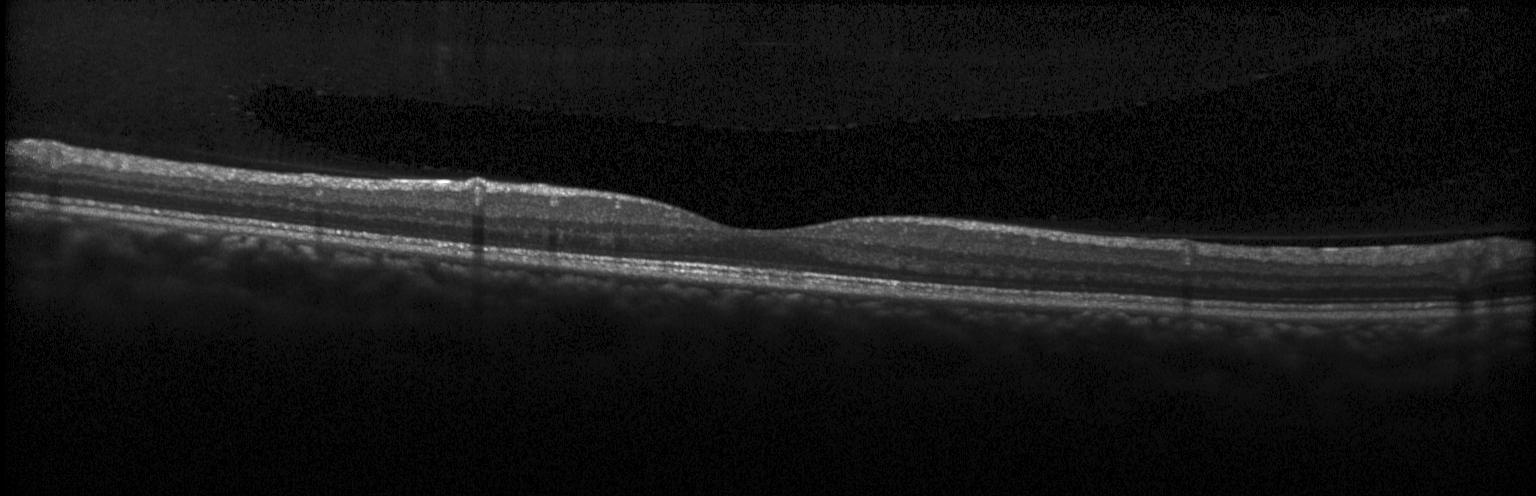

Instrument: Heidelberg Spectralis; optical coherence tomography B-scan. Finding: no evidence of CNV, DME, or drusen.